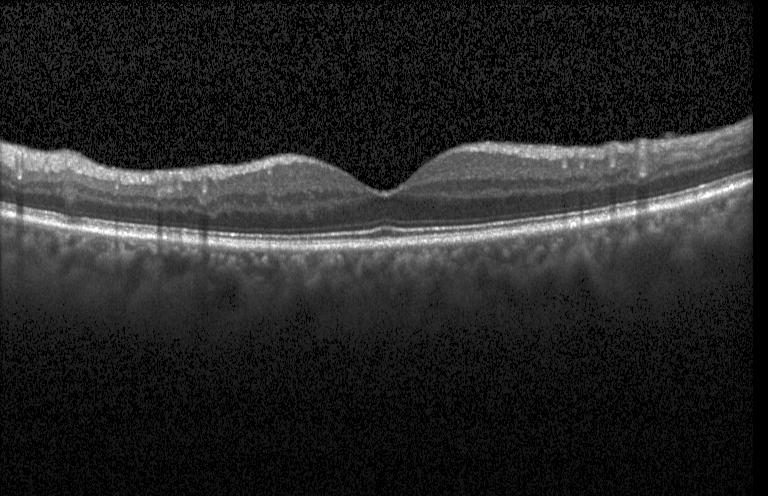

Retinal OCT cross-section, spectral-domain optical coherence tomography — No choroidal neovascularization, diabetic macular edema, or drusen.